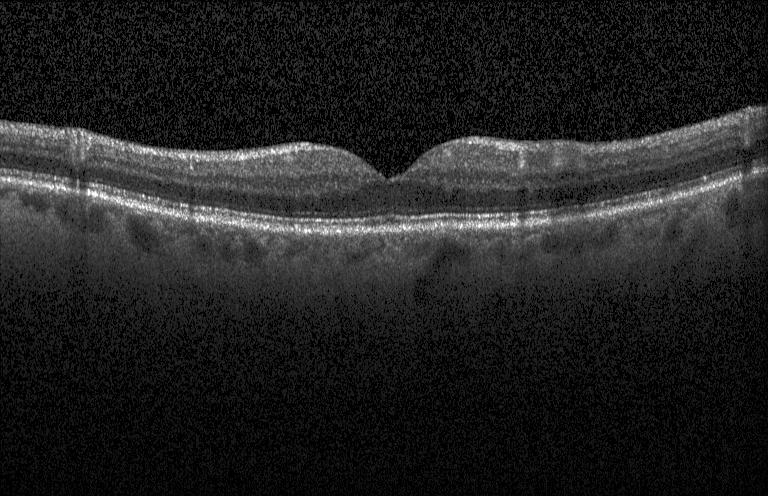

Spectral-domain OCT, retinal OCT B-scan, centered on the fovea. Impression: no evidence of choroidal neovascularization, diabetic macular edema, or drusen.